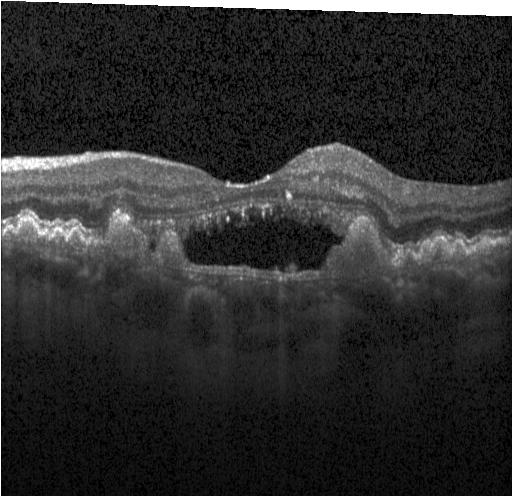 Dx: CNV.